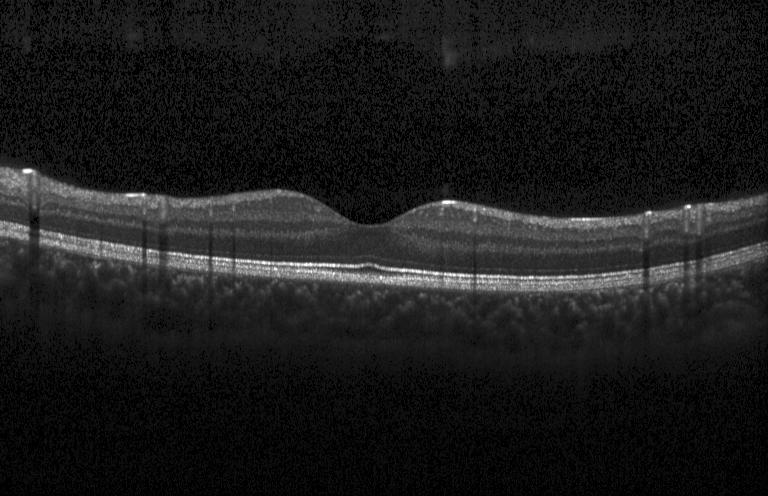

Retinal OCT B-scan — Diagnosis: no CNV, DME, or drusen.